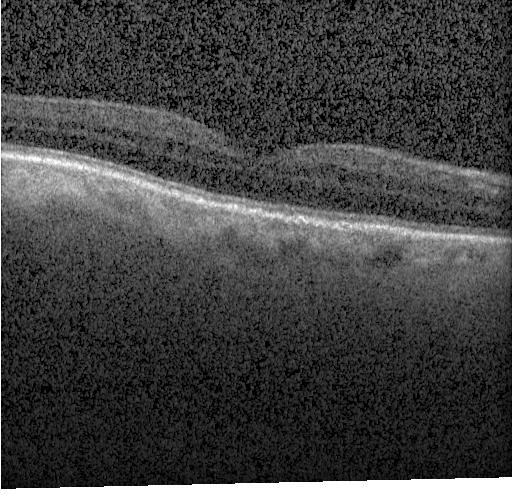 OCT finding: no CNV, no DME, and no drusen.